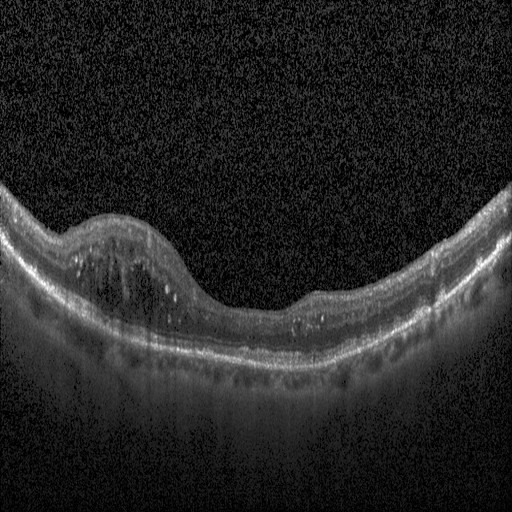
Spectral-domain OCT B-scan: DME.